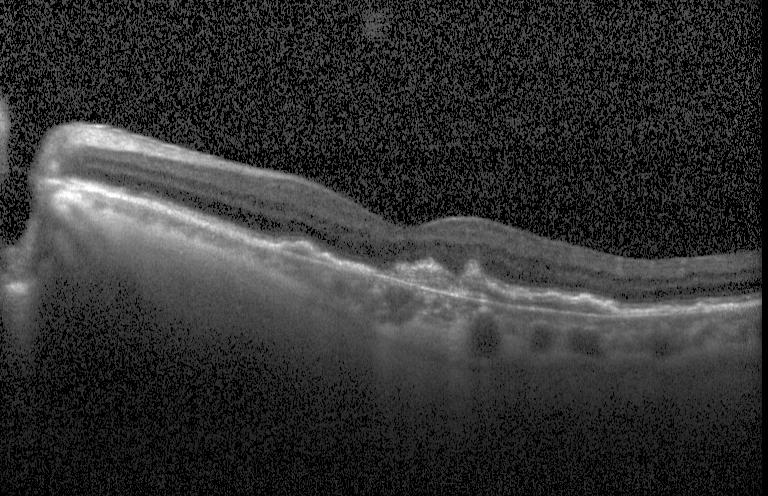 Diagnosis: a choroidal neovascular membrane.